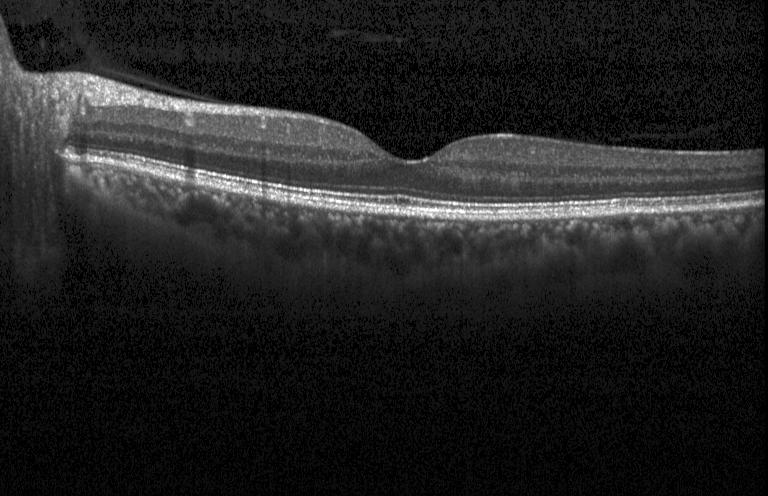

Retinal OCT cross-section · spectral-domain optical coherence tomography
Macular OCT: no evidence of CNV, DME, or drusen.